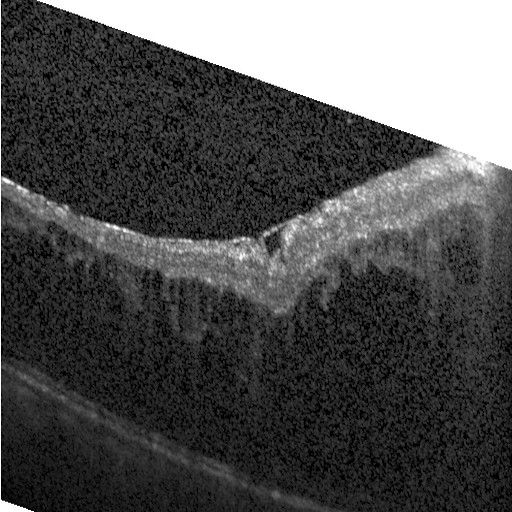 OCT line scan
Macular OCT: DME.